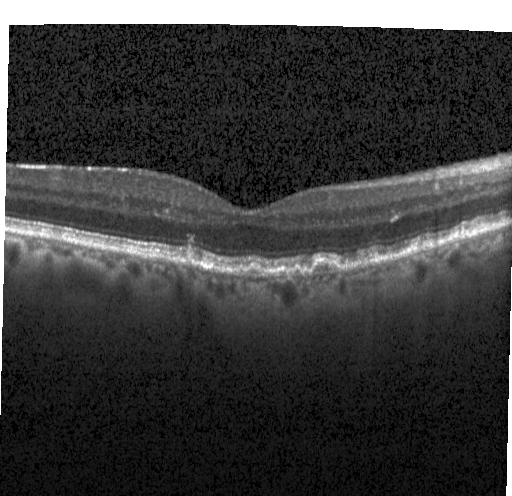
Spectral-domain OCT B-scan: multiple drusen.